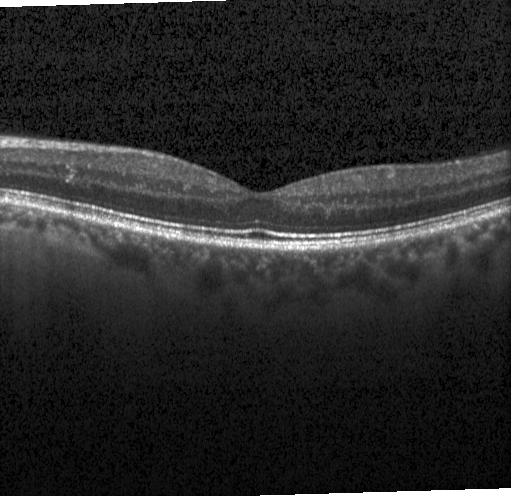
Diagnosis: no choroidal neovascularization, no diabetic macular edema, and no drusen.